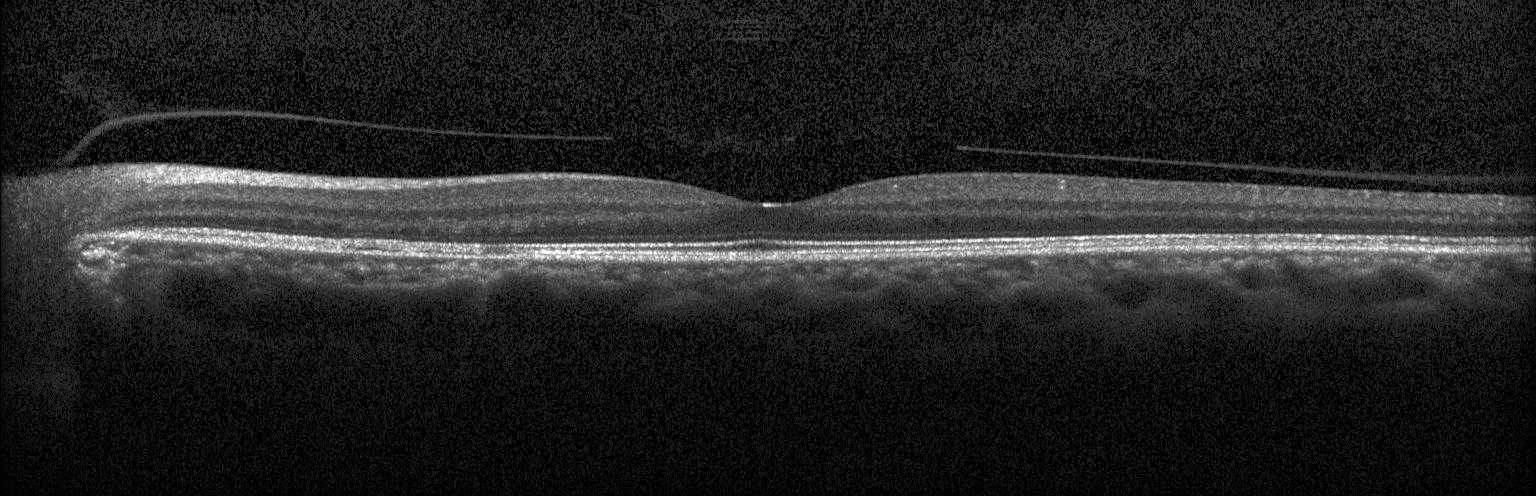
Spectral-domain optical coherence tomography, OCT line scan
Neither choroidal neovascularization, diabetic macular edema, nor drusen.